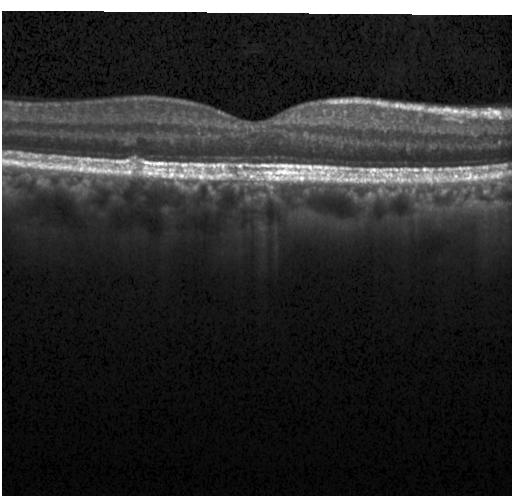 Acquired on a Heidelberg Spectralis, macular scan, optical coherence tomography B-scan.
Finding: sub-RPE drusenoid deposits.